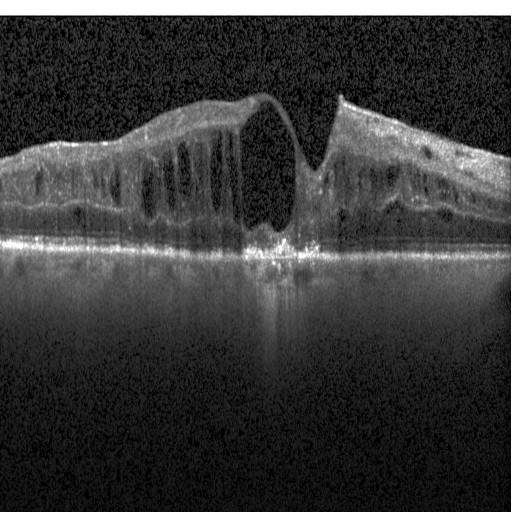

The scan shows diabetic macular edema.